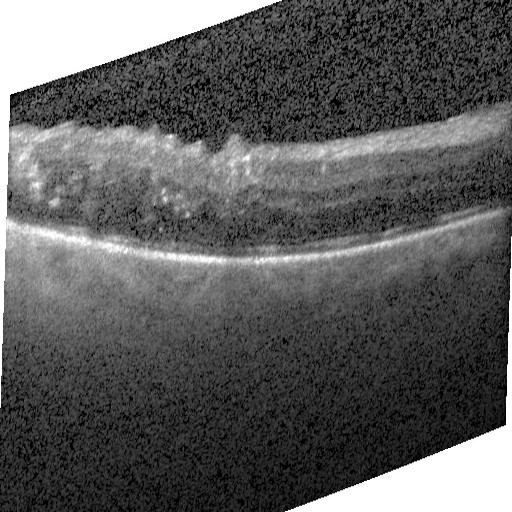

Macular scan. SD-OCT. Optical coherence tomography B-scan
Diagnosis: diabetic macular edema.